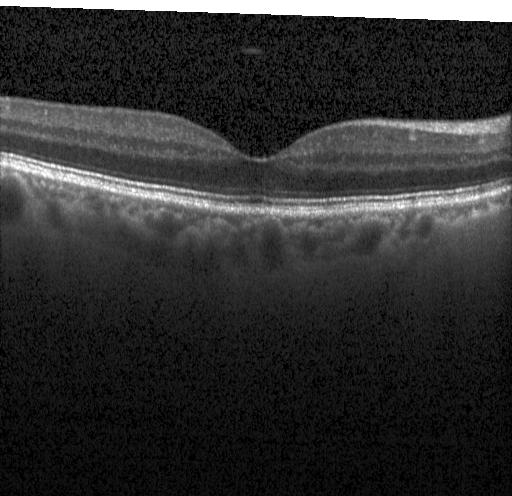
OCT finding: no CNV, DME, or drusen.